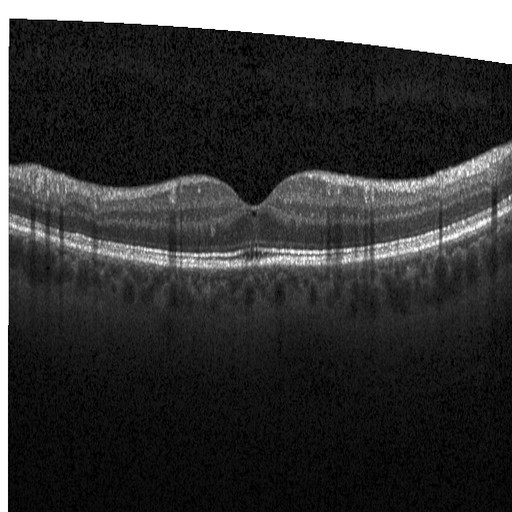 The scan shows DME.